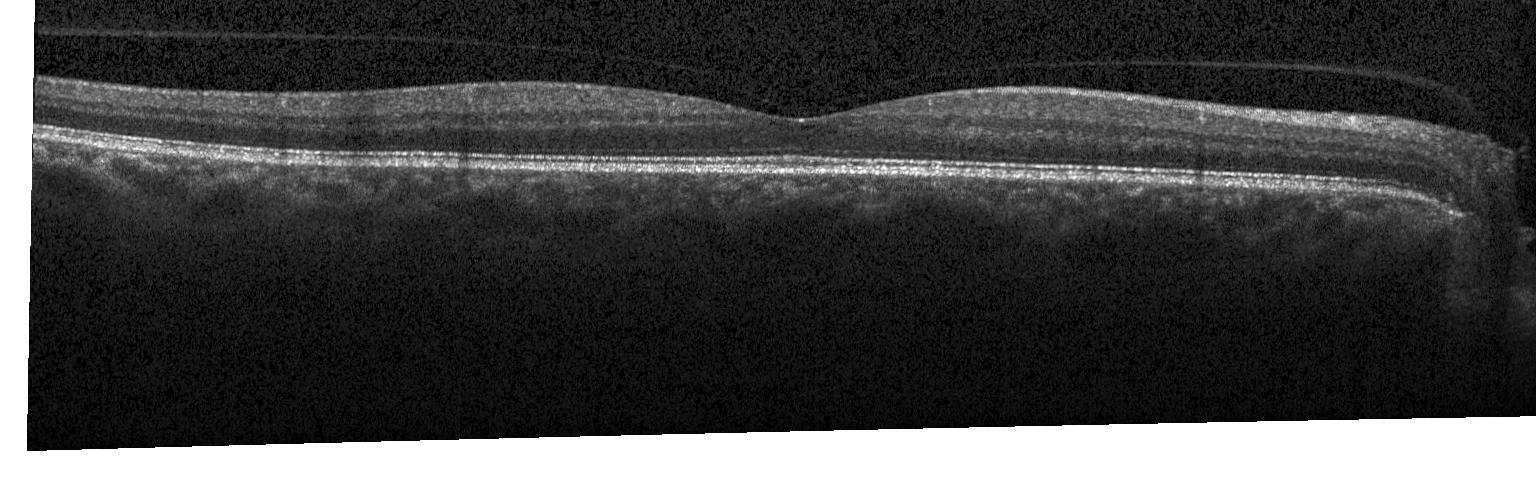 SD-OCT, OCT B-scan, instrument: Heidelberg Spectralis, through the macula — Diagnosis: no choroidal neovascularization, diabetic macular edema, or drusen.